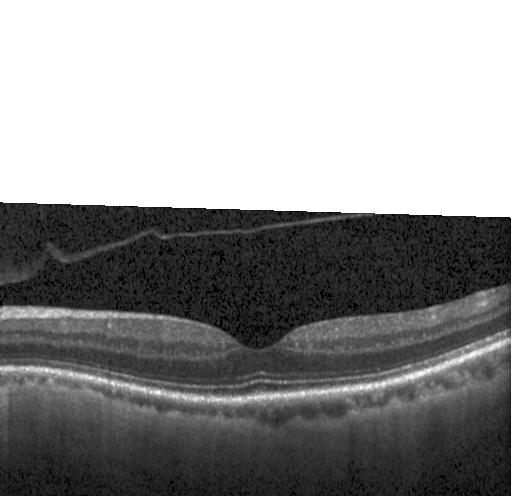 OCT line scan.
Finding: no evidence of CNV, DME, or drusen.